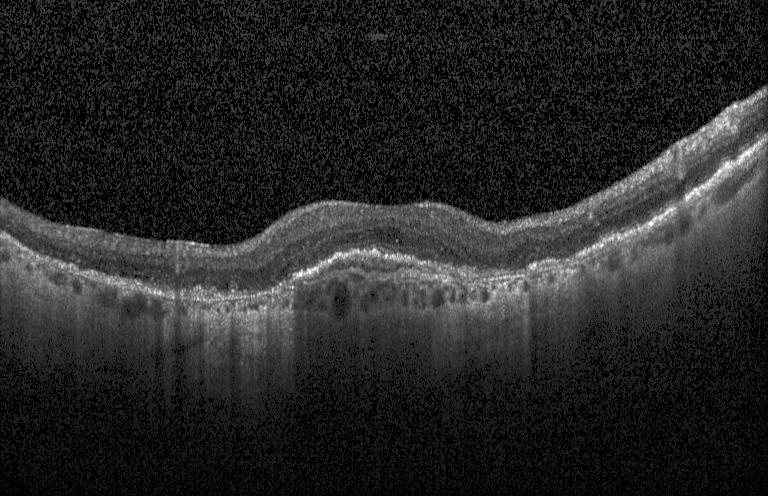

Heidelberg Spectralis; optical coherence tomography B-scan; spectral-domain optical coherence tomography. Finding: CNV.